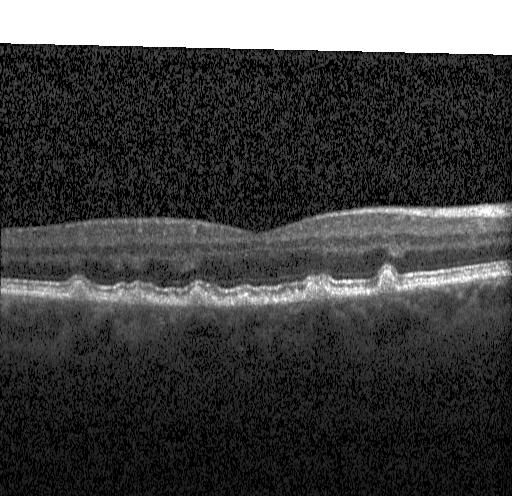 Centered on the fovea. Optical coherence tomography scan — Multiple drusen.